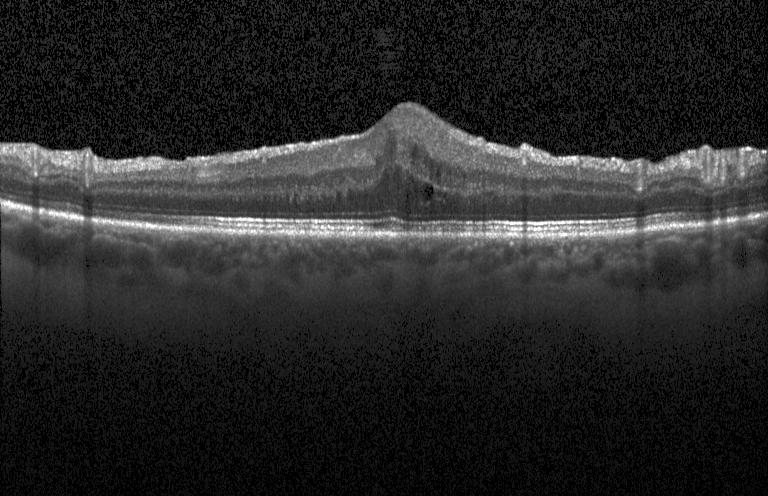
Retinal OCT cross-section.
This B-scan demonstrates diabetic macular edema (DME).